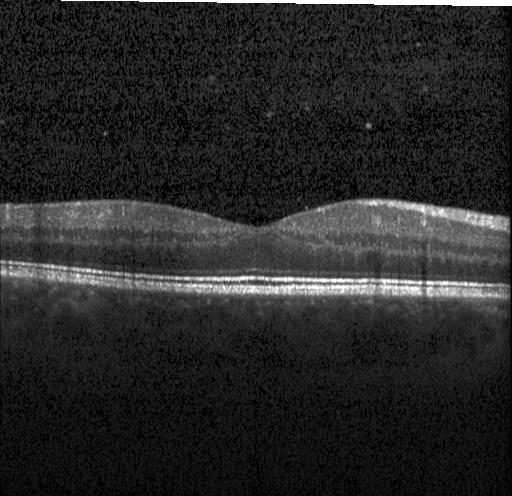

Spectral-domain optical coherence tomography. Centered on the fovea. OCT B-scan
Finding: no evidence of choroidal neovascularization, diabetic macular edema, or drusen.